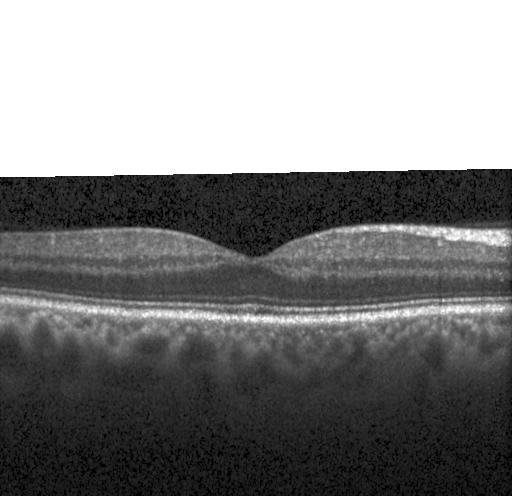 Impression: neither CNV, DME, nor drusen.